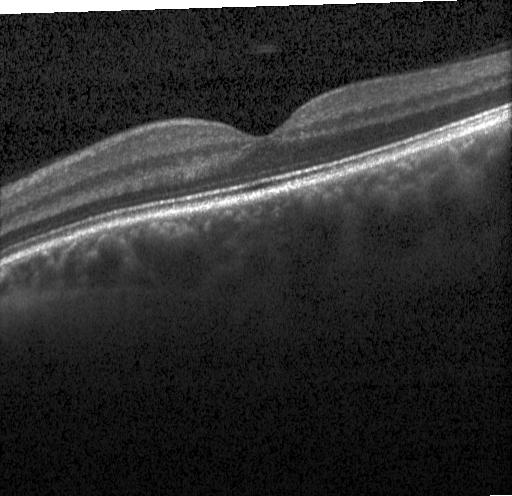

Dx: neither choroidal neovascularization, diabetic macular edema, nor drusen.